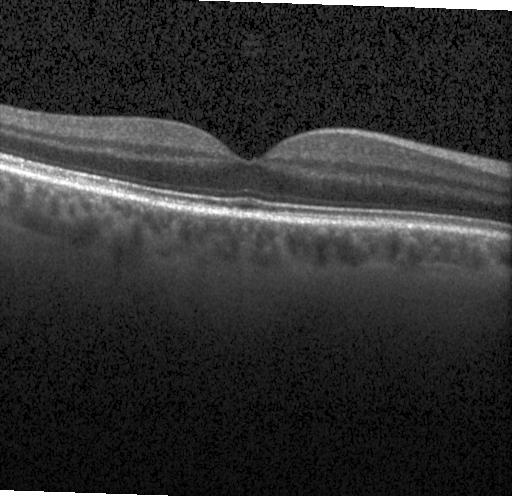
OCT line scan
This B-scan demonstrates neither choroidal neovascularization, diabetic macular edema, nor drusen.